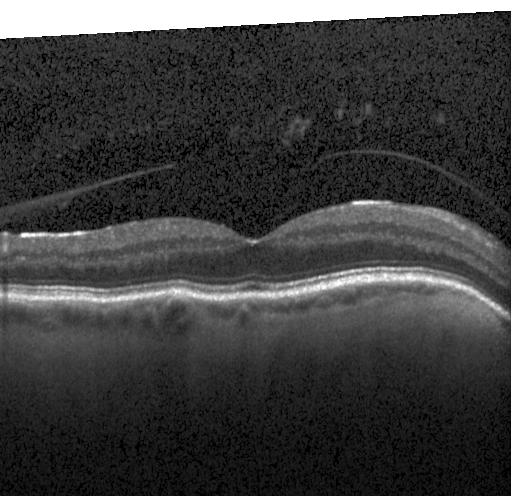
Retinal OCT B-scan
Finding: no CNV, DME, or drusen.